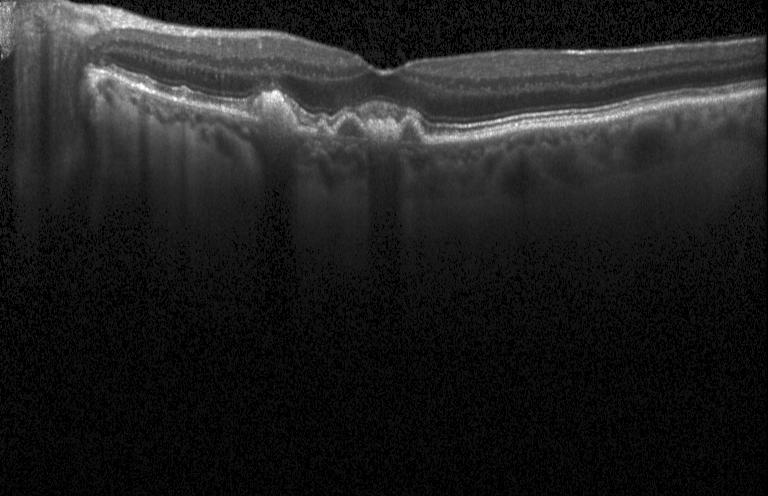
Macular scan · SD-OCT · optical coherence tomography B-scan · Heidelberg Spectralis OCT system
Diagnosis: choroidal neovascularization (CNV).